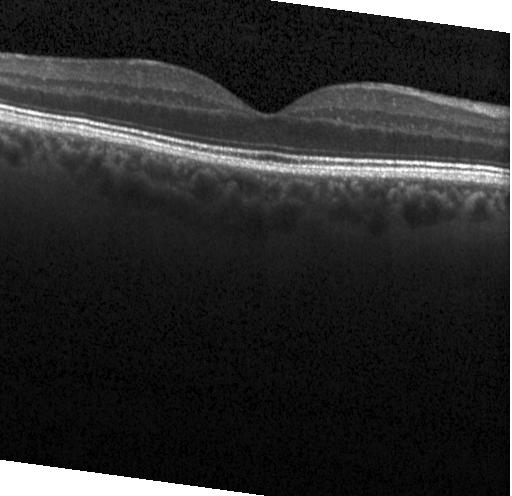 Instrument: Heidelberg Spectralis, optical coherence tomography B-scan, macular scan, spectral-domain optical coherence tomography. Diagnosis: no choroidal neovascularization, no diabetic macular edema, and no drusen.